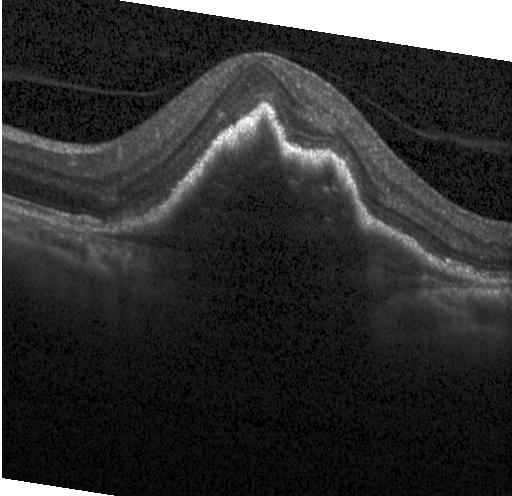 Heidelberg Spectralis. Optical coherence tomography B-scan. CNV.